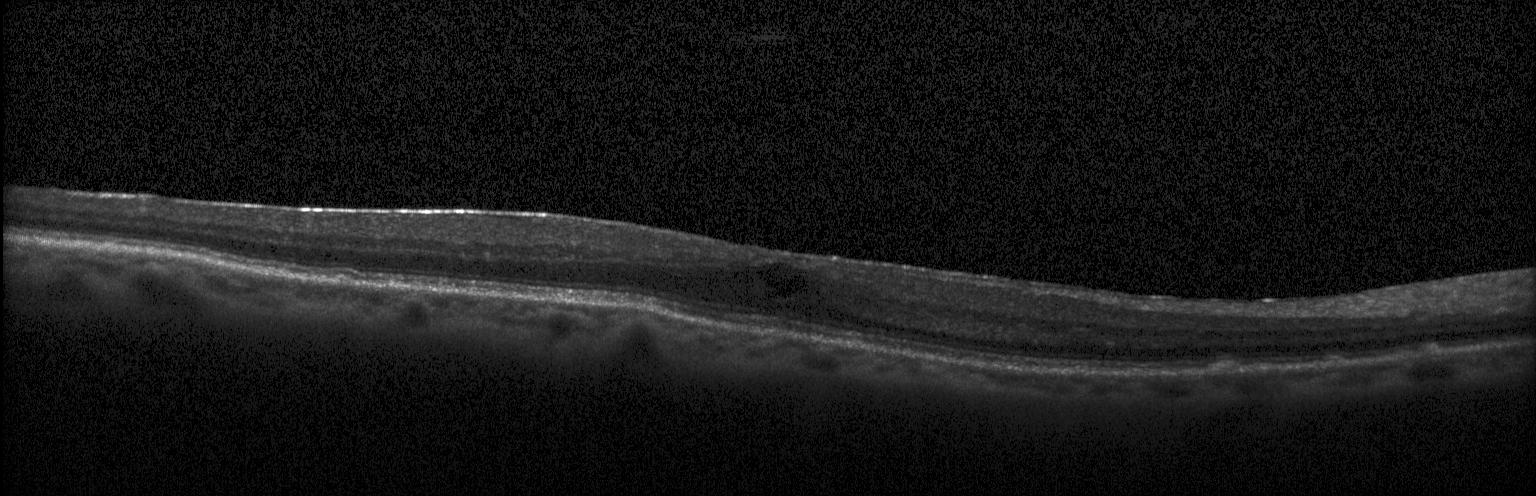 Retinal OCT cross-section, Heidelberg Spectralis OCT system, centered on the fovea, spectral-domain optical coherence tomography — Diabetic macular edema.